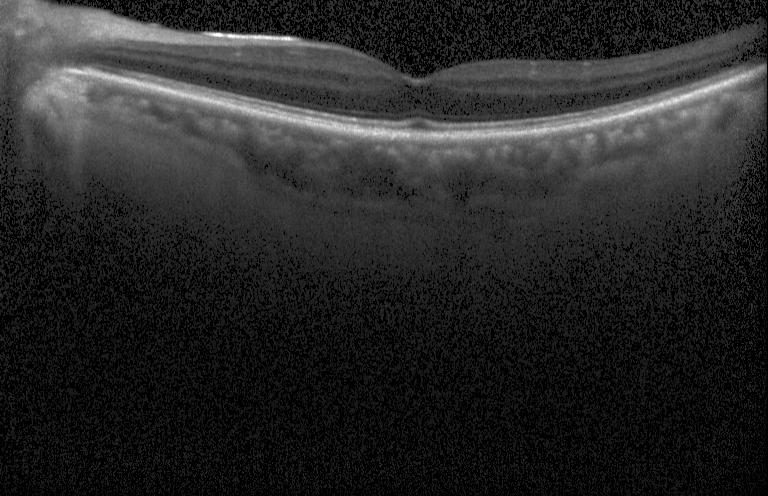
Retinal OCT cross-section. Acquired on a Heidelberg Spectralis. Spectral-domain OCT. Fovea-centered
Diagnosis: neither choroidal neovascularization, diabetic macular edema, nor drusen.